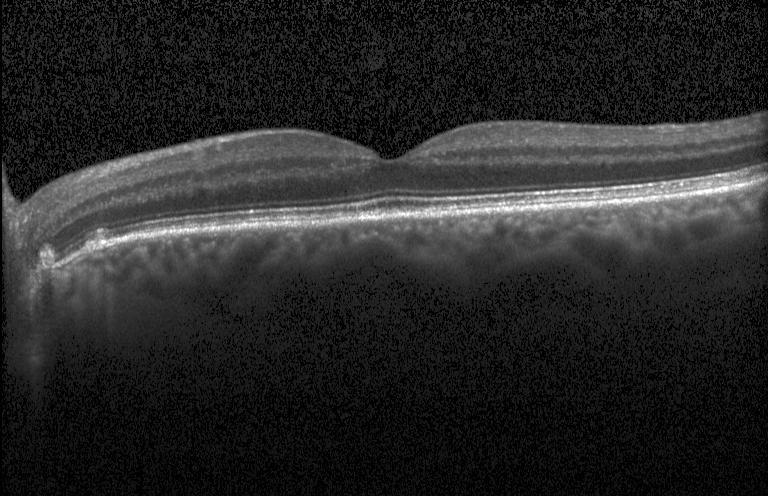

Retinal OCT B-scan · spectral-domain OCT · through the macula · acquired on a Heidelberg Spectralis — Dx: no CNV, no DME, and no drusen.